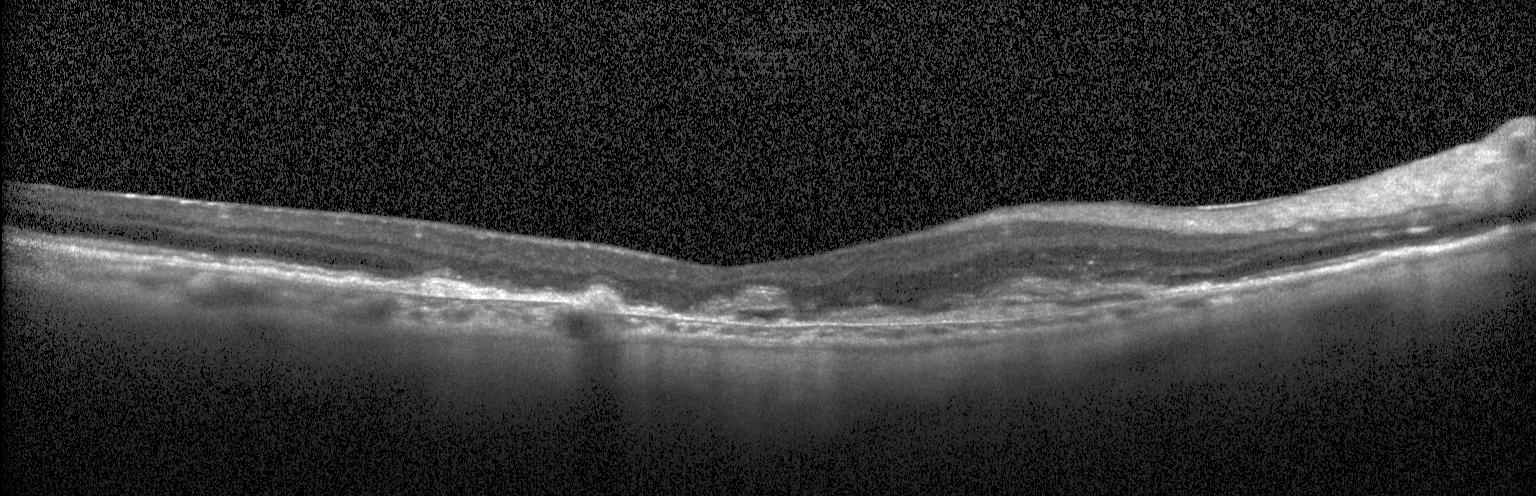
Retinal OCT cross-section, spectral-domain optical coherence tomography, Heidelberg Spectralis OCT system
Diagnosis: CNV.